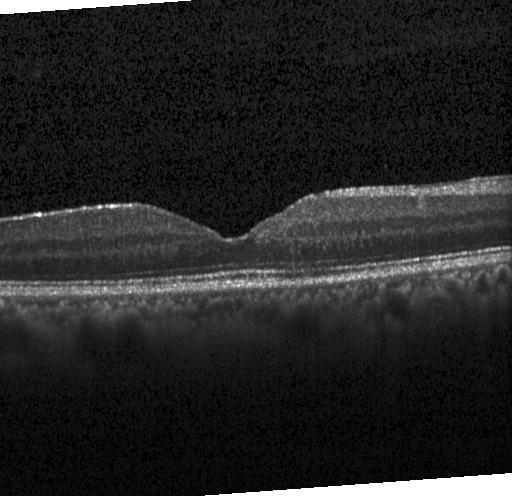

Macular OCT: no evidence of choroidal neovascularization, diabetic macular edema, or drusen.